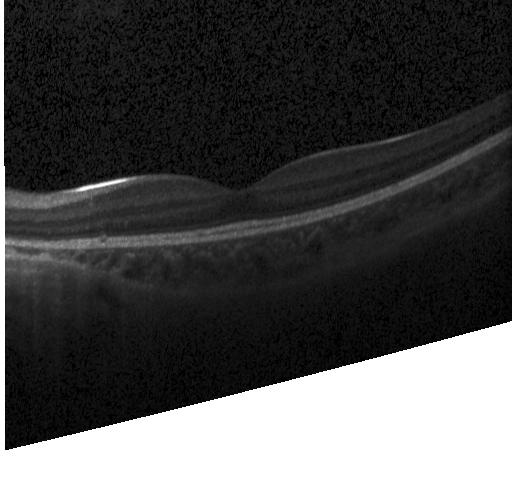
Optical coherence tomography B-scan; Heidelberg Spectralis — Dx: no CNV, no DME, and no drusen.